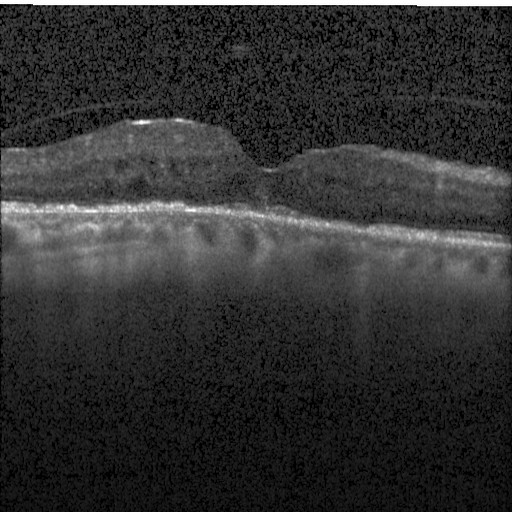

This B-scan demonstrates DME.